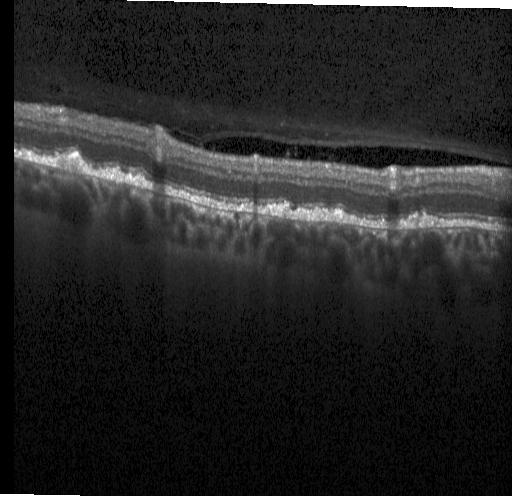

Diagnosis: multiple drusen.